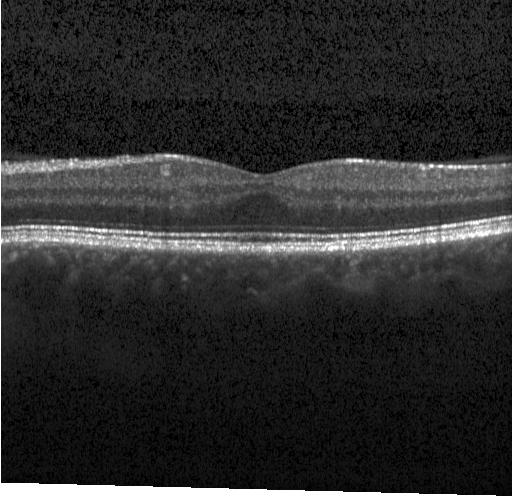

Horizontal scan through the fovea; instrument: Heidelberg Spectralis; optical coherence tomography B-scan.
This B-scan demonstrates neither CNV, DME, nor drusen.